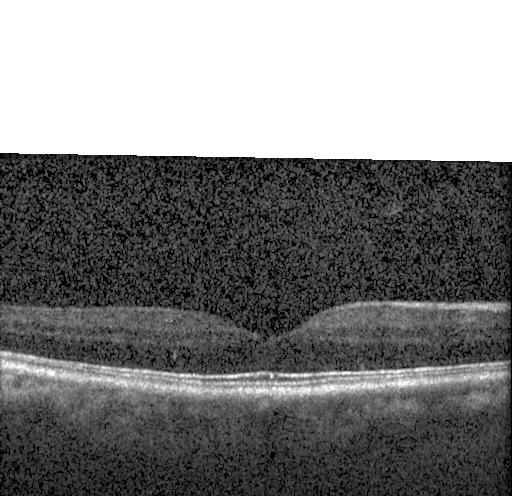
Macular OCT: no evidence of choroidal neovascularization, diabetic macular edema, or drusen.